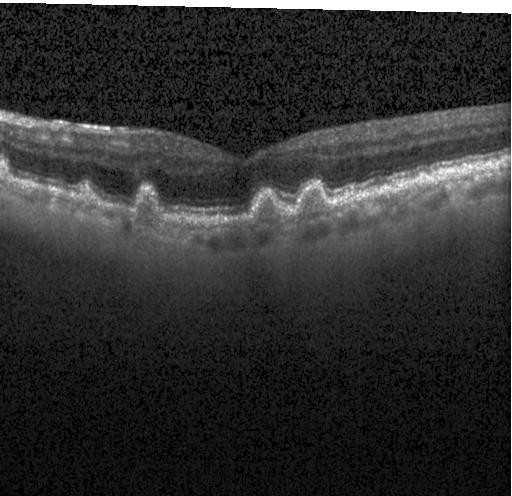 Centered on the fovea. Heidelberg Spectralis. Spectral-domain OCT. Optical coherence tomography scan. Finding: sub-RPE drusenoid deposits.